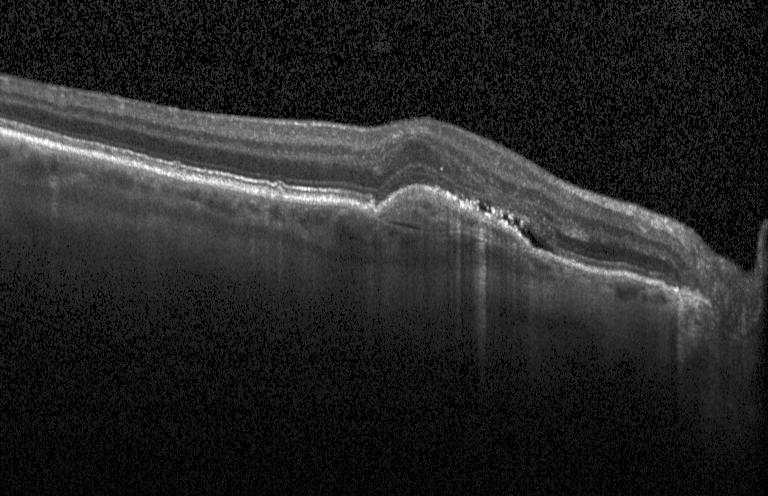 Retinal OCT cross-section showing choroidal neovascularization (CNV).